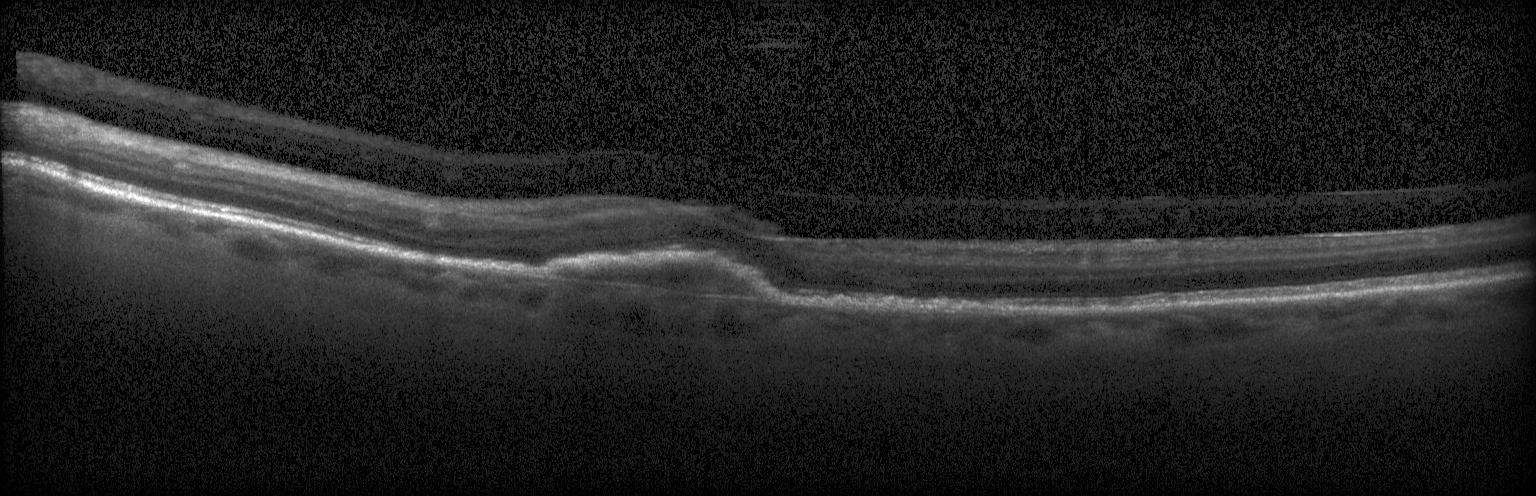
Retinal OCT B-scan; centered on the fovea; spectral-domain optical coherence tomography; Heidelberg Spectralis. Finding: a choroidal neovascular membrane.